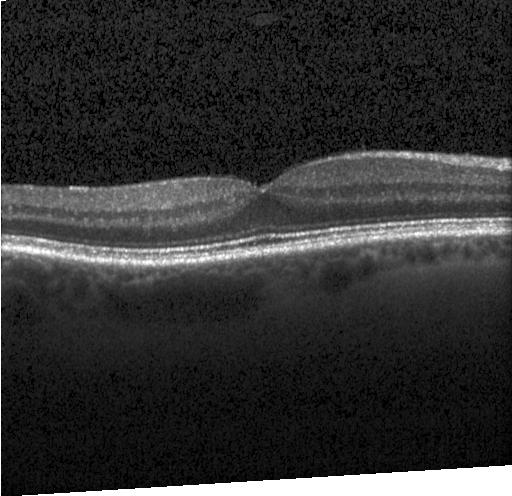

Retinal OCT cross-section showing no evidence of choroidal neovascularization, diabetic macular edema, or drusen.